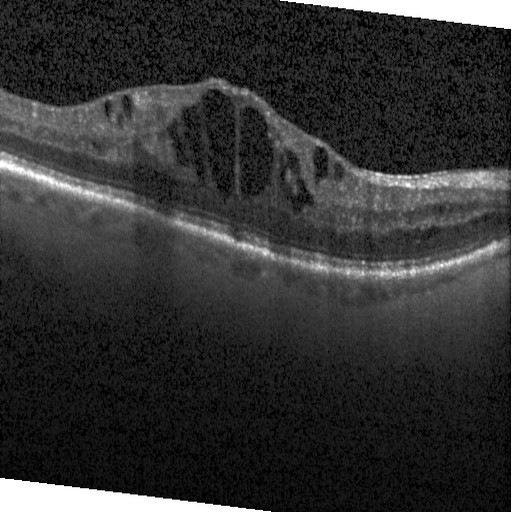 This B-scan demonstrates diabetic macular edema (DME).